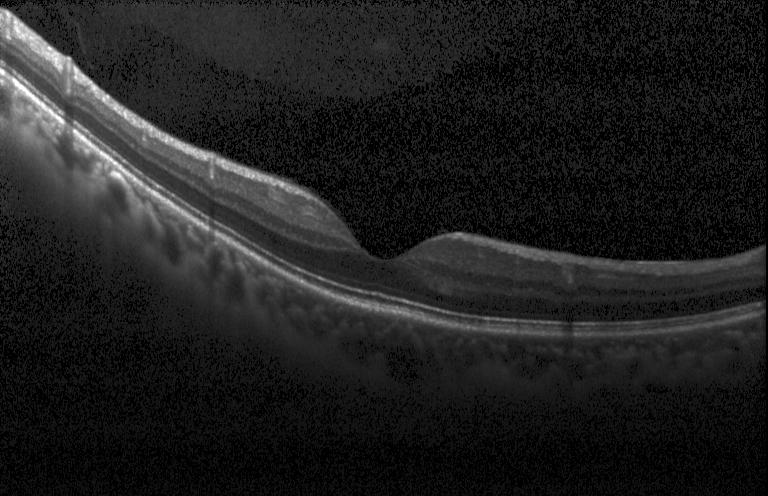

Impression: no choroidal neovascularization, no diabetic macular edema, and no drusen.